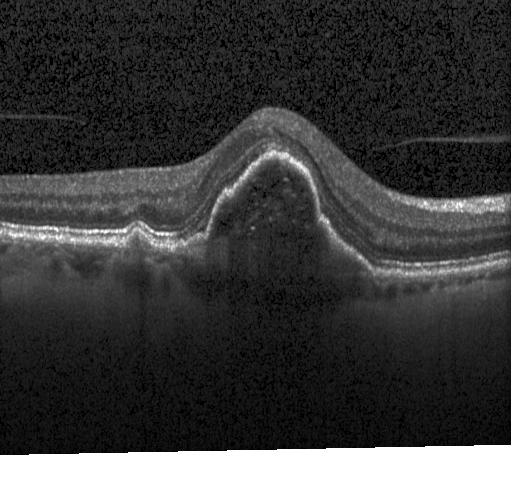 Retinal OCT cross-section
Diagnosis: choroidal neovascularization.